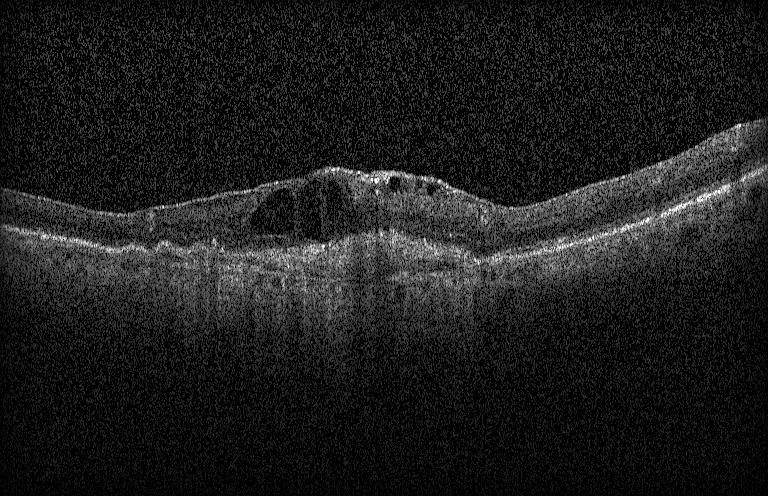 Optical coherence tomography B-scan — Diagnosis: a choroidal neovascular membrane.